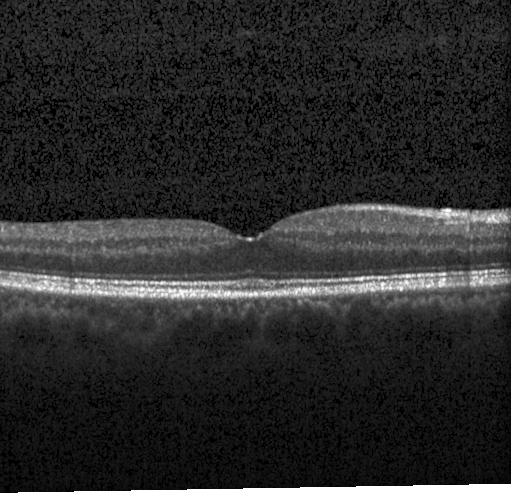 Retinal OCT cross-section showing no CNV, no DME, and no drusen.